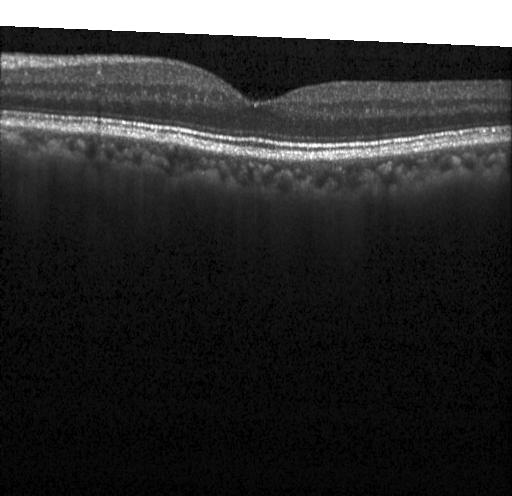 Retinal OCT B-scan.
Finding: neither choroidal neovascularization, diabetic macular edema, nor drusen.